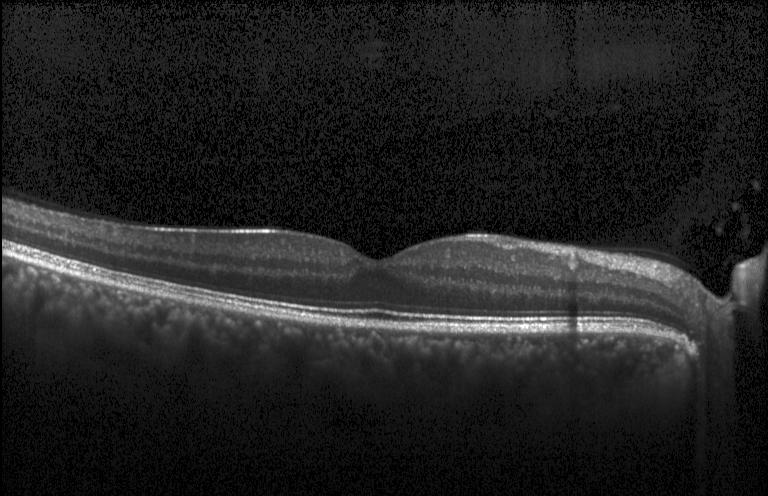 Optical coherence tomography scan. Heidelberg Spectralis. Through the macula. Macular OCT: neither choroidal neovascularization, diabetic macular edema, nor drusen.